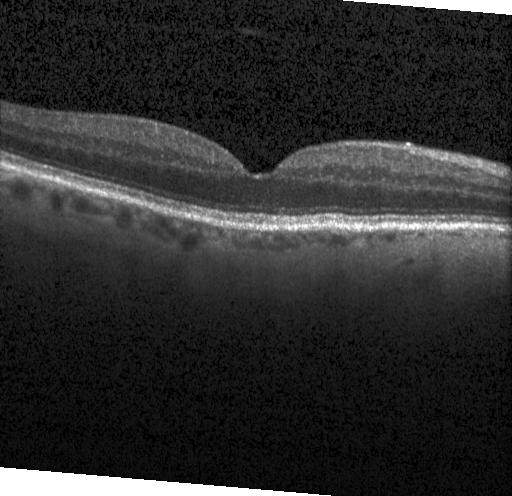

Retinal OCT B-scan — OCT finding: no choroidal neovascularization, diabetic macular edema, or drusen.